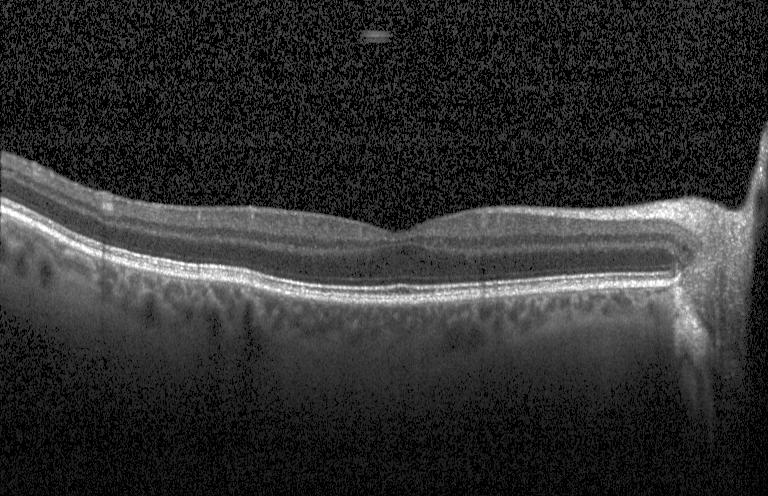

OCT B-scan. Centered on the fovea. Diagnosis: no CNV, DME, or drusen.